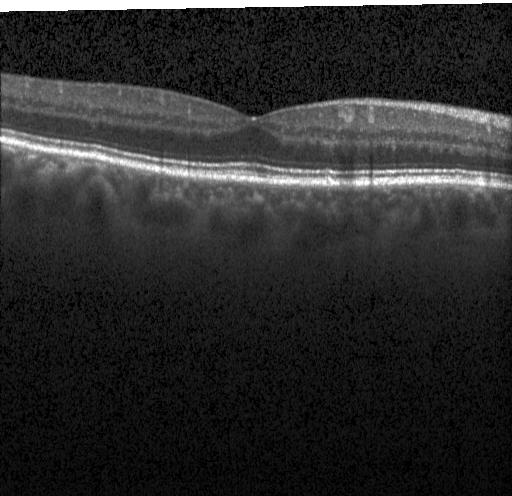
No choroidal neovascularization, no diabetic macular edema, and no drusen.